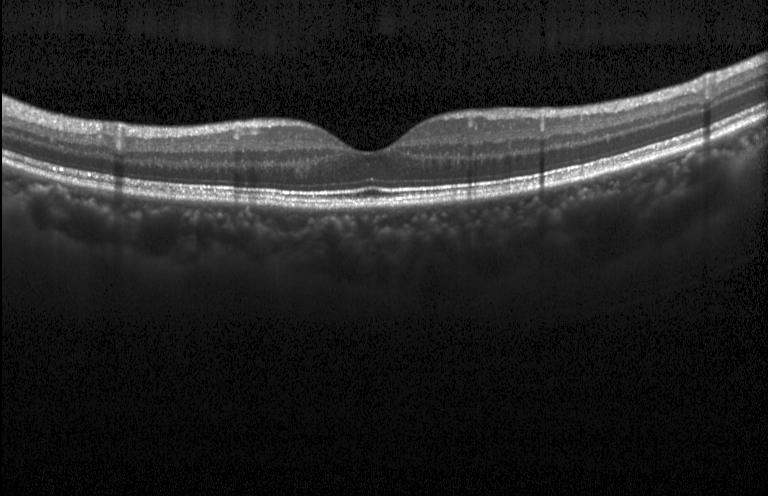 Through the macula, retinal OCT B-scan
Diagnosis: no choroidal neovascularization, no diabetic macular edema, and no drusen.